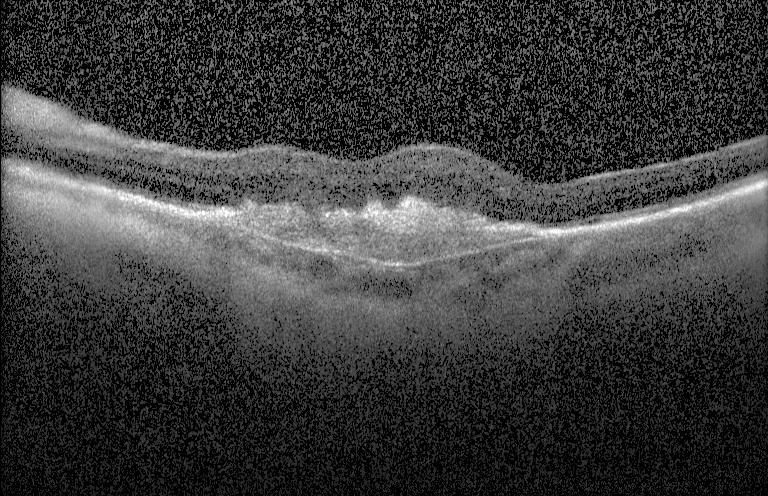 Retinal OCT B-scan. Through the macula. Heidelberg Spectralis. Finding: choroidal neovascularization.